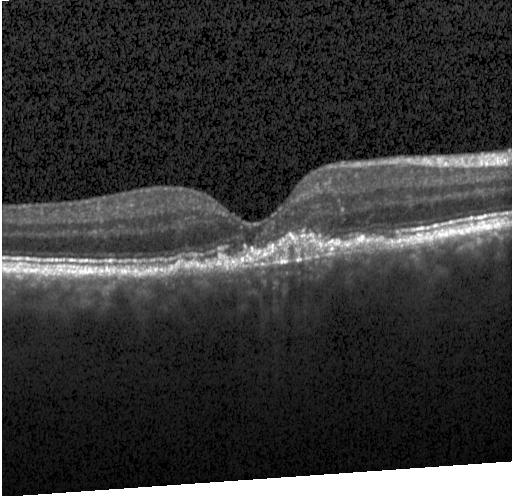 A choroidal neovascular membrane.